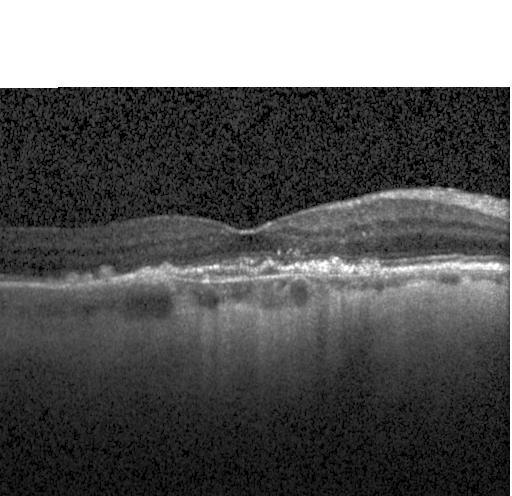

Acquired on a Heidelberg Spectralis · optical coherence tomography B-scan. Impression: a choroidal neovascular membrane.